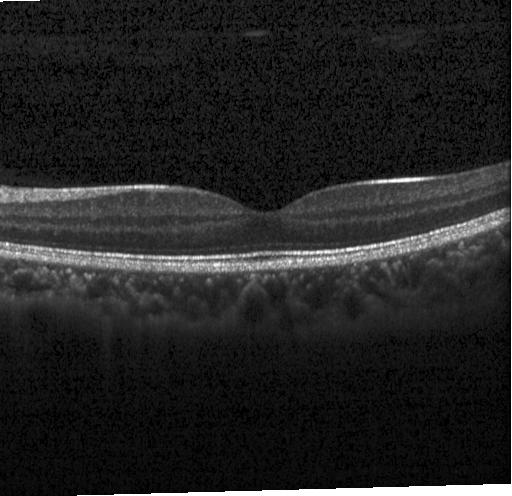

Finding: no evidence of choroidal neovascularization, diabetic macular edema, or drusen.